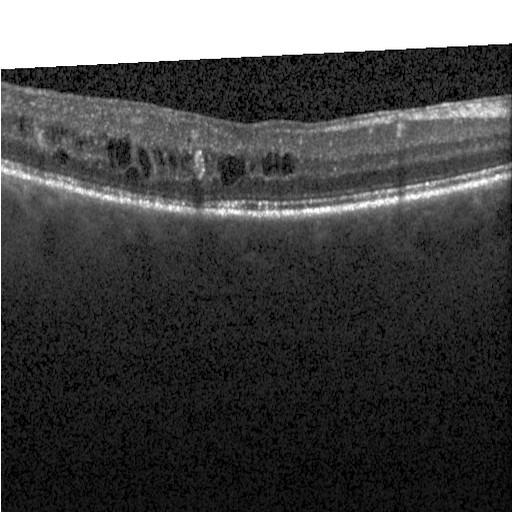
OCT line scan.
Impression: diabetic macular edema.